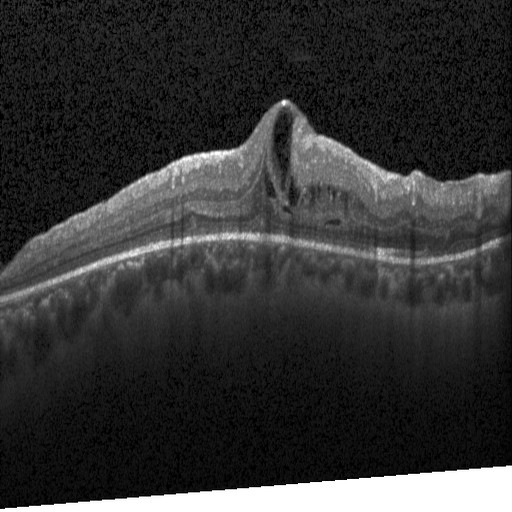

OCT line scan
Finding: DME.